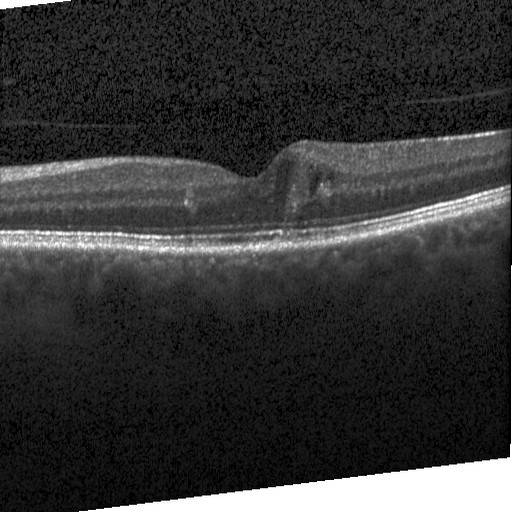

Retinal OCT cross-section · SD-OCT.
Assessment: DME.